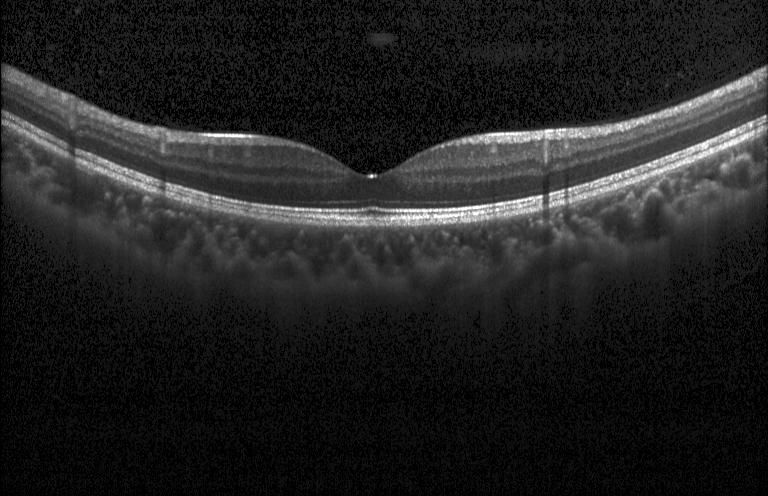

Macular OCT: neither CNV, DME, nor drusen.